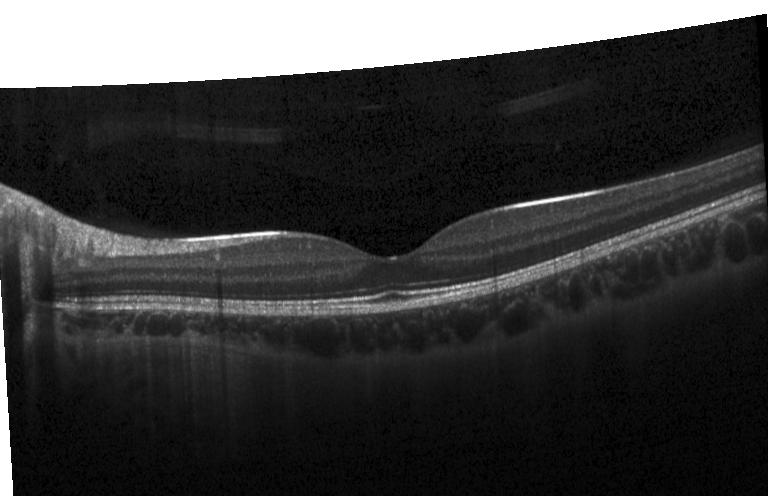
Retinal OCT cross-section. Centered on the fovea — OCT finding: no choroidal neovascularization, no diabetic macular edema, and no drusen.